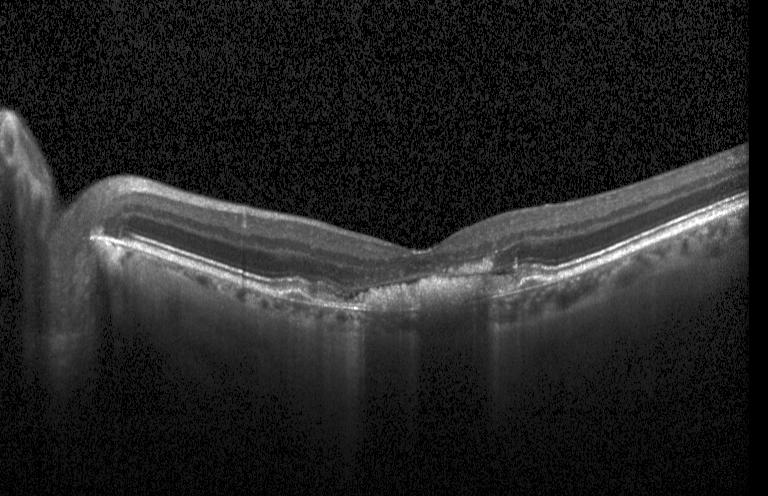 OCT B-scan; spectral-domain optical coherence tomography; centered on the fovea.
The scan shows a choroidal neovascular membrane.